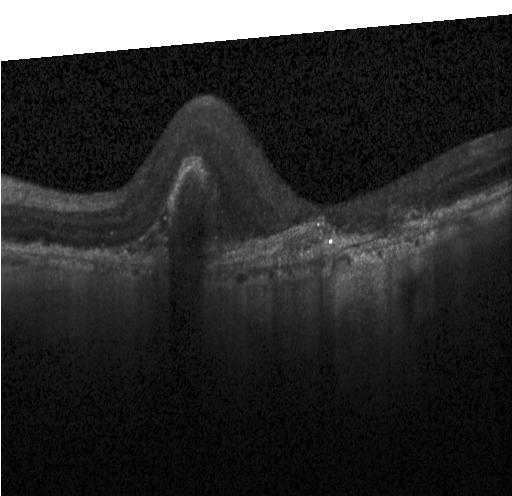 OCT line scan. This B-scan demonstrates choroidal neovascularization (CNV).